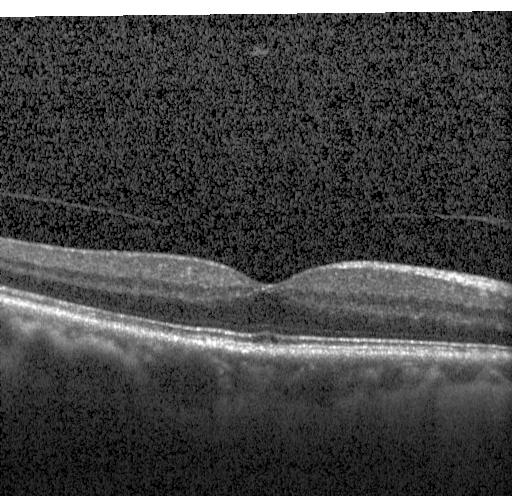

OCT finding: no CNV, no DME, and no drusen.